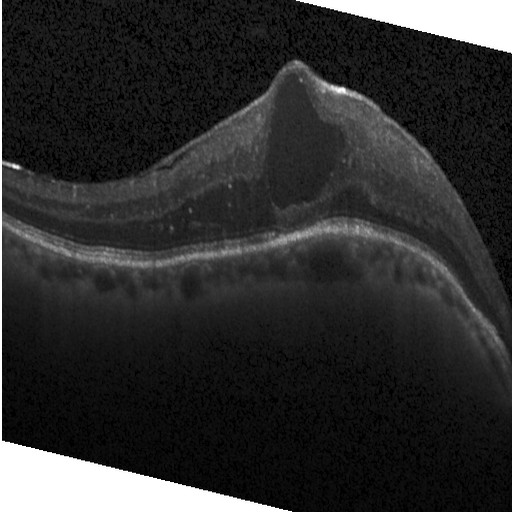 Centered on the fovea; acquired on a Heidelberg Spectralis; retinal OCT cross-section; spectral-domain optical coherence tomography. Diabetic macular edema.